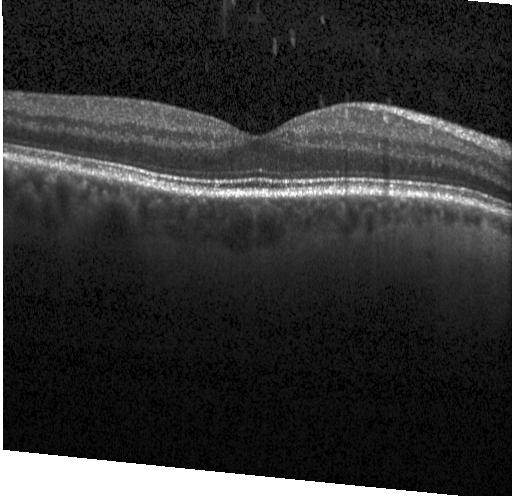
OCT B-scan showing no choroidal neovascularization, diabetic macular edema, or drusen.